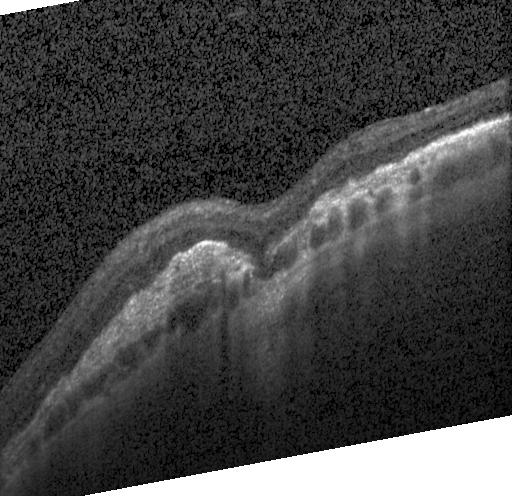

Finding: choroidal neovascularization (CNV).